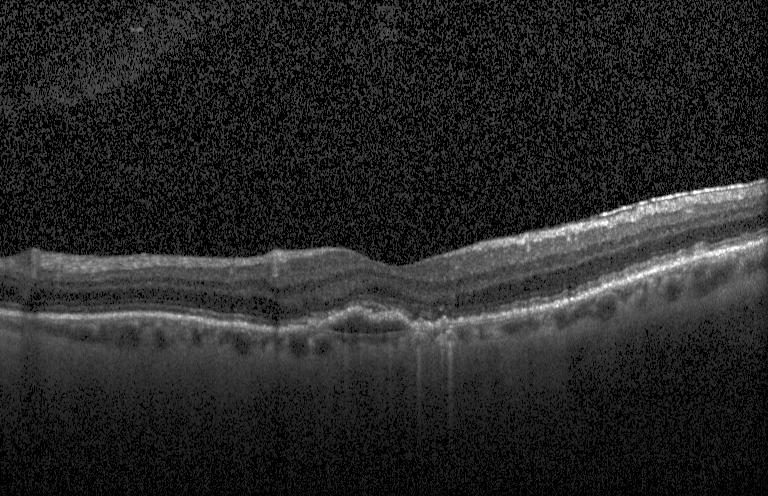
Optical coherence tomography B-scan — Finding: a choroidal neovascular membrane.